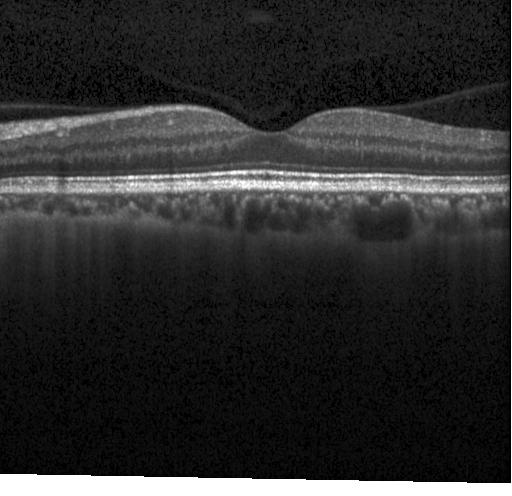 Retinal OCT cross-section showing no evidence of choroidal neovascularization, diabetic macular edema, or drusen.